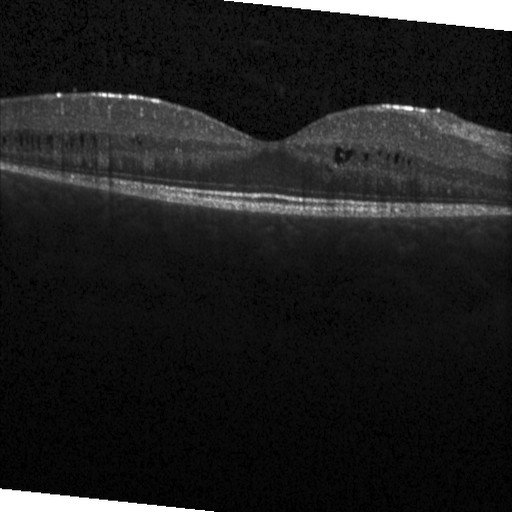 OCT line scan.
Diagnosis: DME.